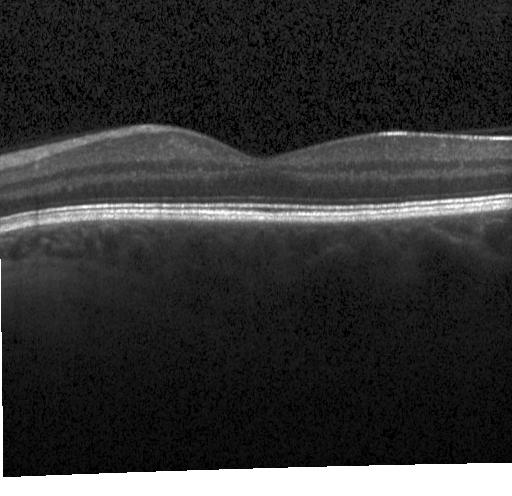 Heidelberg Spectralis · fovea-centered · OCT B-scan.
Impression: neither choroidal neovascularization, diabetic macular edema, nor drusen.